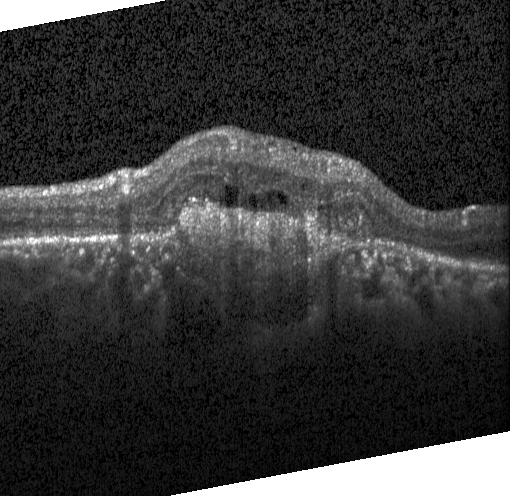
Impression: CNV.